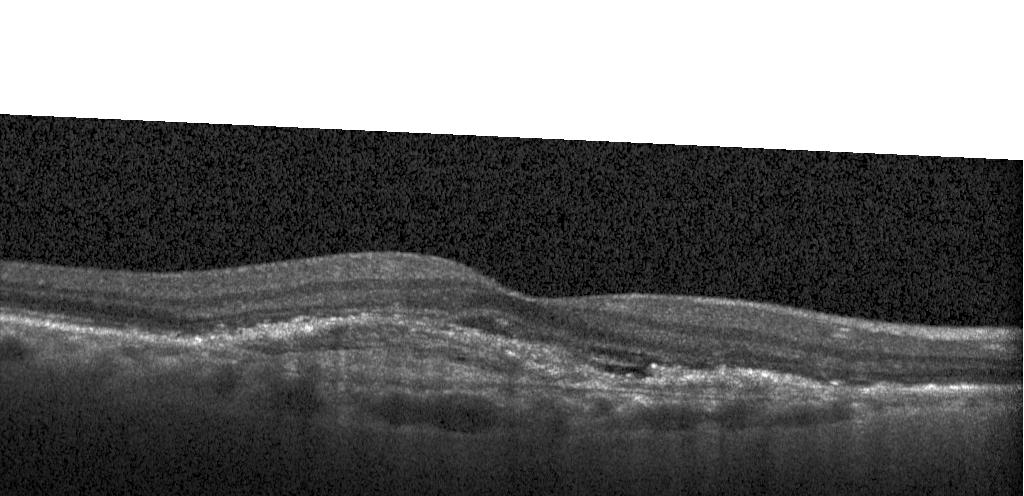
The scan shows a choroidal neovascular membrane.